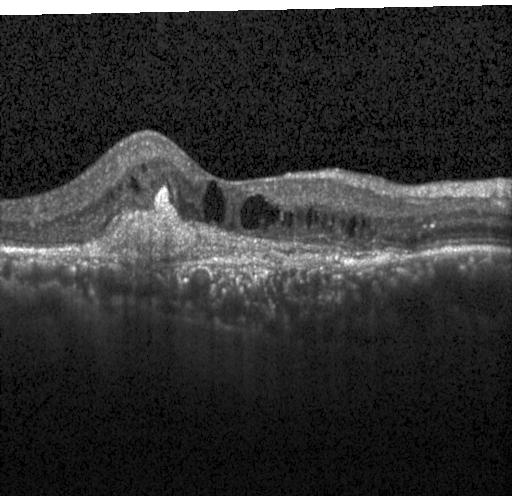

OCT B-scan
Assessment: a choroidal neovascular membrane.